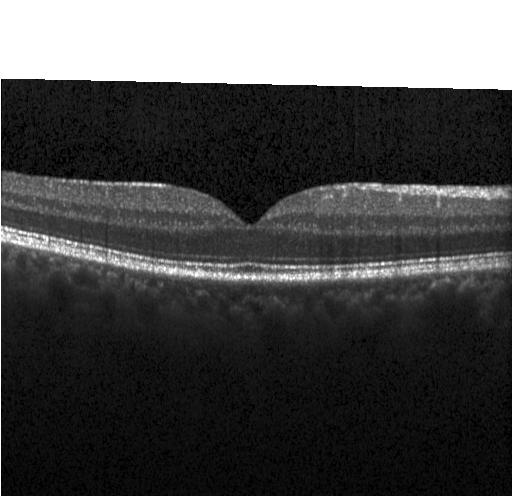 OCT line scan
Impression: neither choroidal neovascularization, diabetic macular edema, nor drusen.